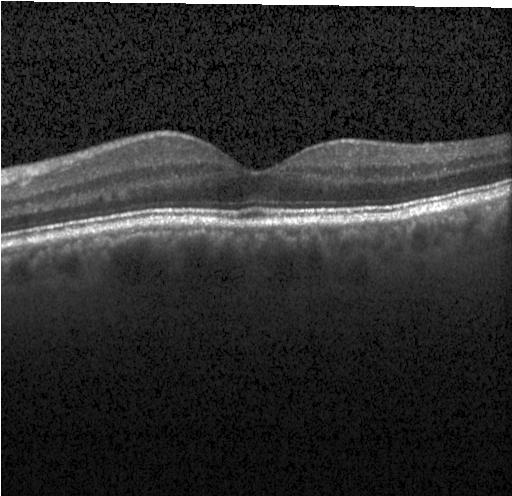

Centered on the fovea, OCT B-scan, SD-OCT, Heidelberg Spectralis
No choroidal neovascularization, no diabetic macular edema, and no drusen.